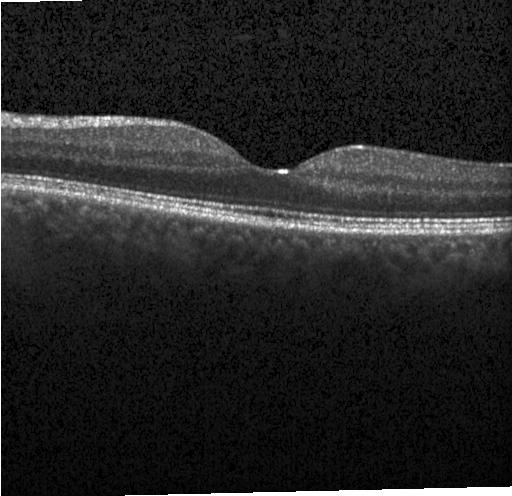
Spectral-domain OCT. OCT line scan.
This B-scan demonstrates no CNV, DME, or drusen.